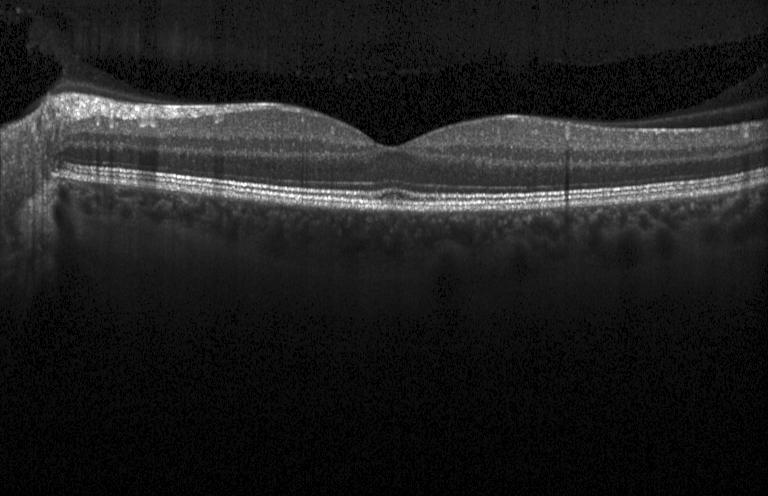 Centered on the fovea, retinal OCT cross-section, instrument: Heidelberg Spectralis, spectral-domain OCT
Diagnosis: no choroidal neovascularization, no diabetic macular edema, and no drusen.